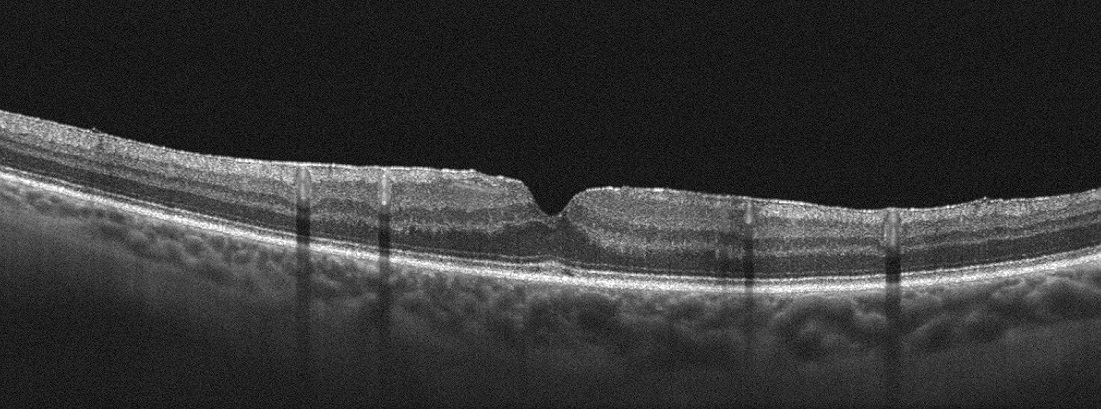 Finding: ERM.